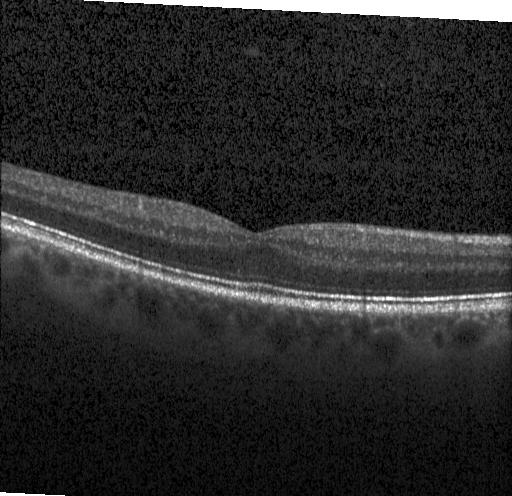 Retinal OCT B-scan · spectral-domain OCT. Impression: no choroidal neovascularization, no diabetic macular edema, and no drusen.